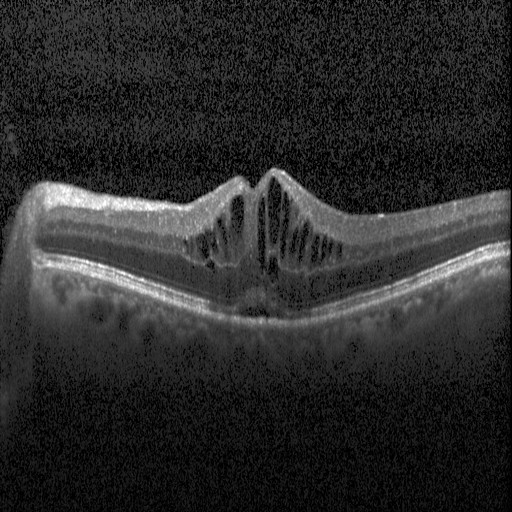
Finding: DME.